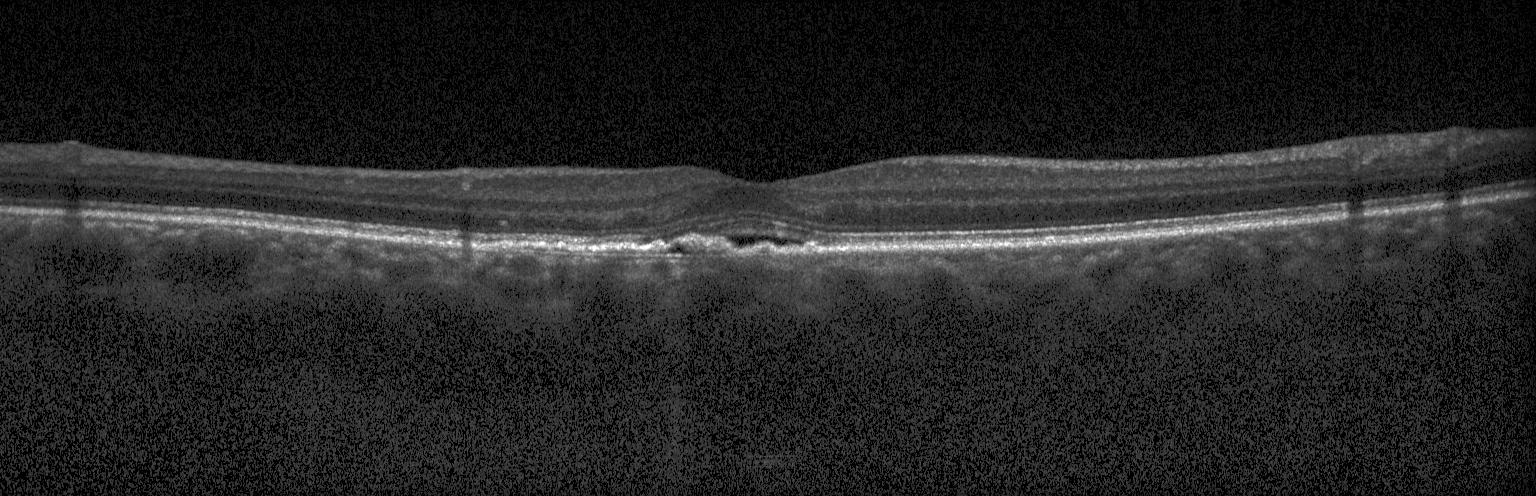

Finding: a choroidal neovascular membrane.